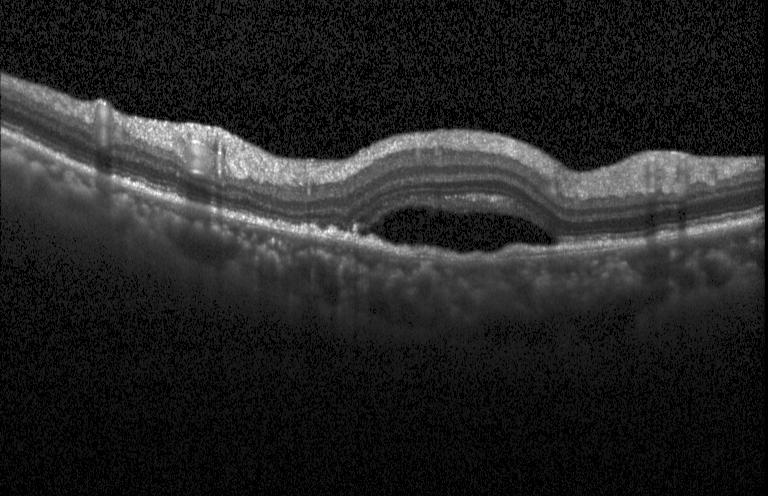
Retinal OCT B-scan — Diagnosis: CNV.